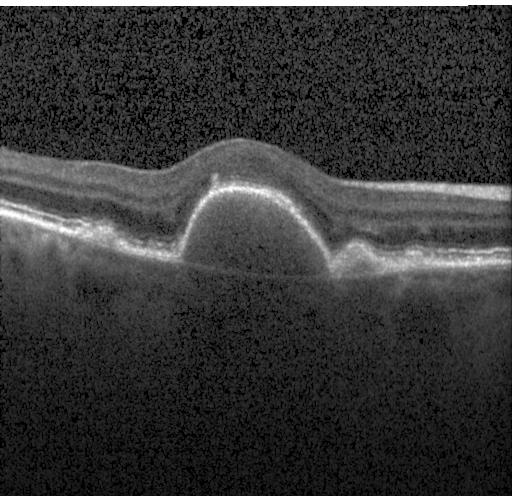 Acquired on a Heidelberg Spectralis, optical coherence tomography B-scan
Assessment: a choroidal neovascular membrane.